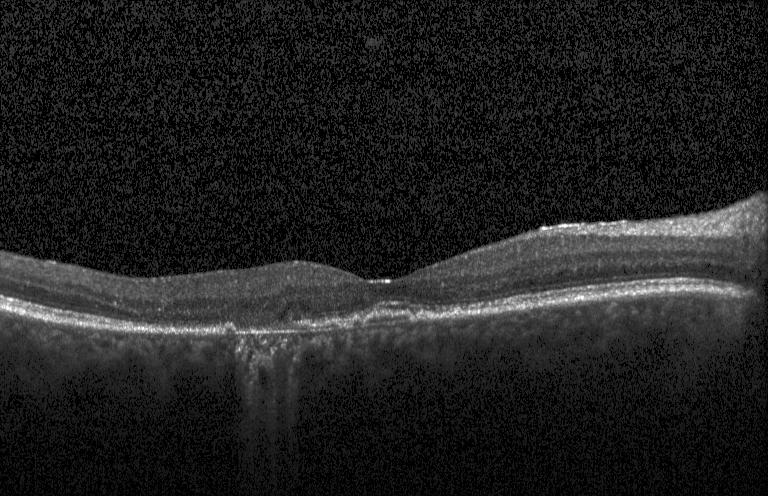
OCT line scan. Through the macula. Spectral-domain optical coherence tomography. Heidelberg Spectralis OCT system. Diagnosis: choroidal neovascularization (CNV).